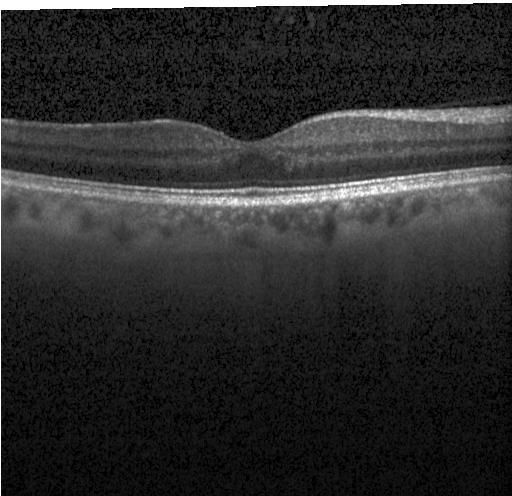
Retinal OCT B-scan. Finding: neither CNV, DME, nor drusen.